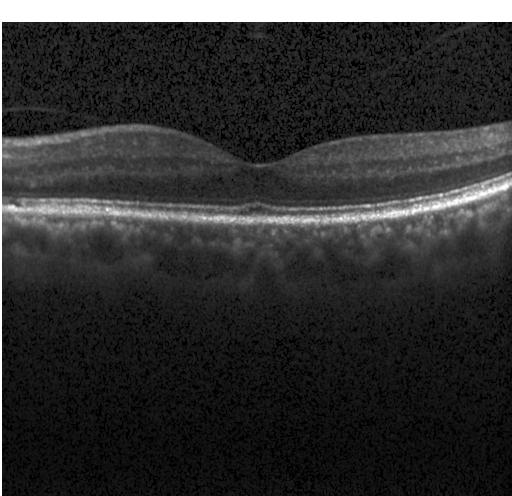
Impression: no evidence of choroidal neovascularization, diabetic macular edema, or drusen.